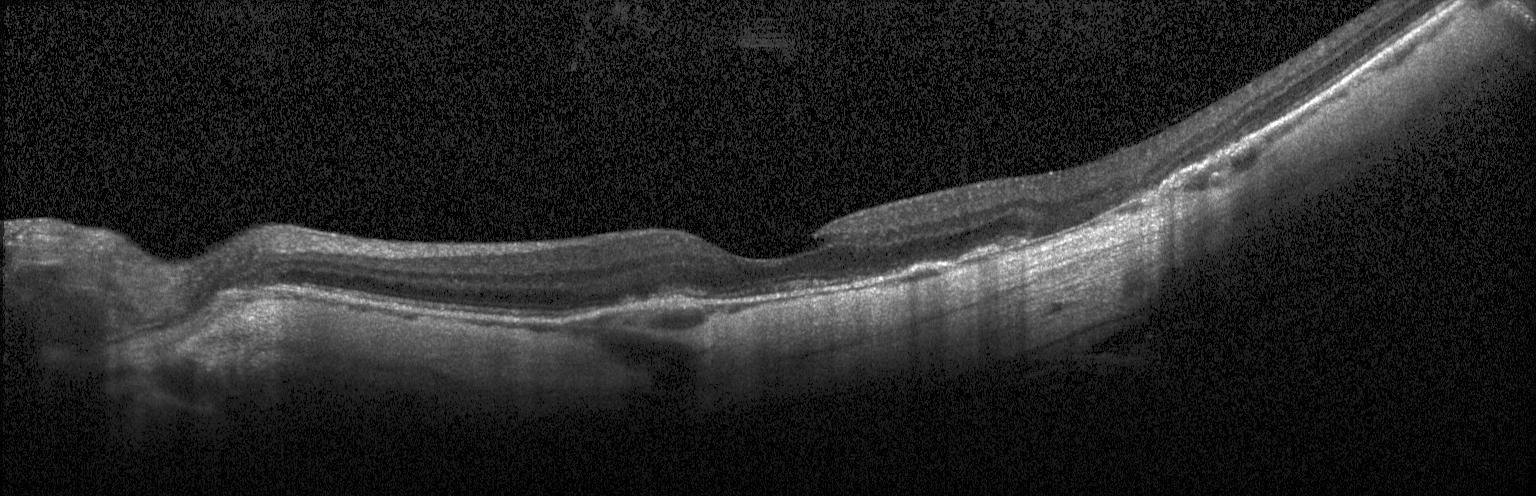

OCT B-scan, macular scan, spectral-domain OCT.
Diagnosis: a choroidal neovascular membrane.